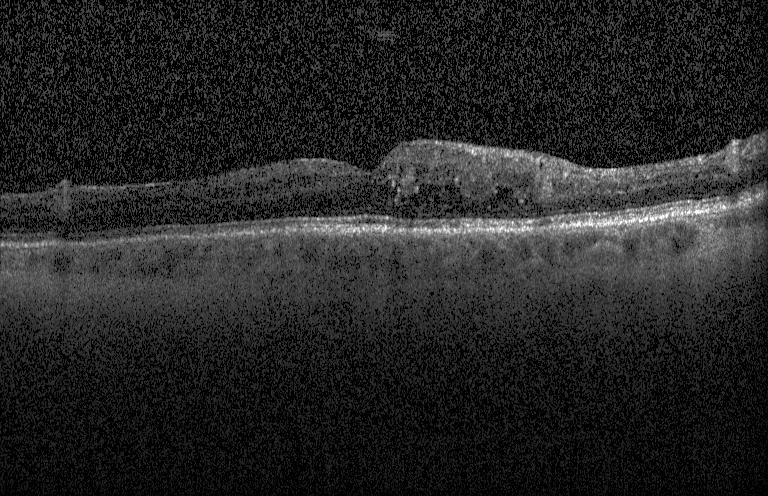

Macular OCT: diabetic macular edema (DME).